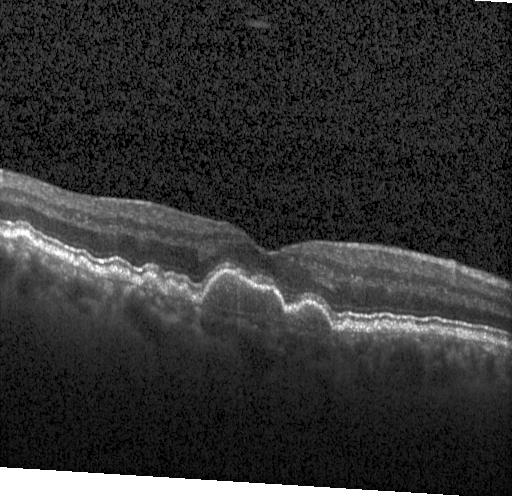

The scan shows drusen.